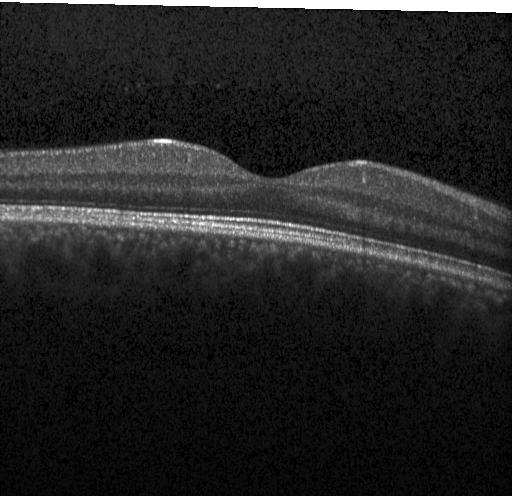
Diagnosis: no choroidal neovascularization, no diabetic macular edema, and no drusen.